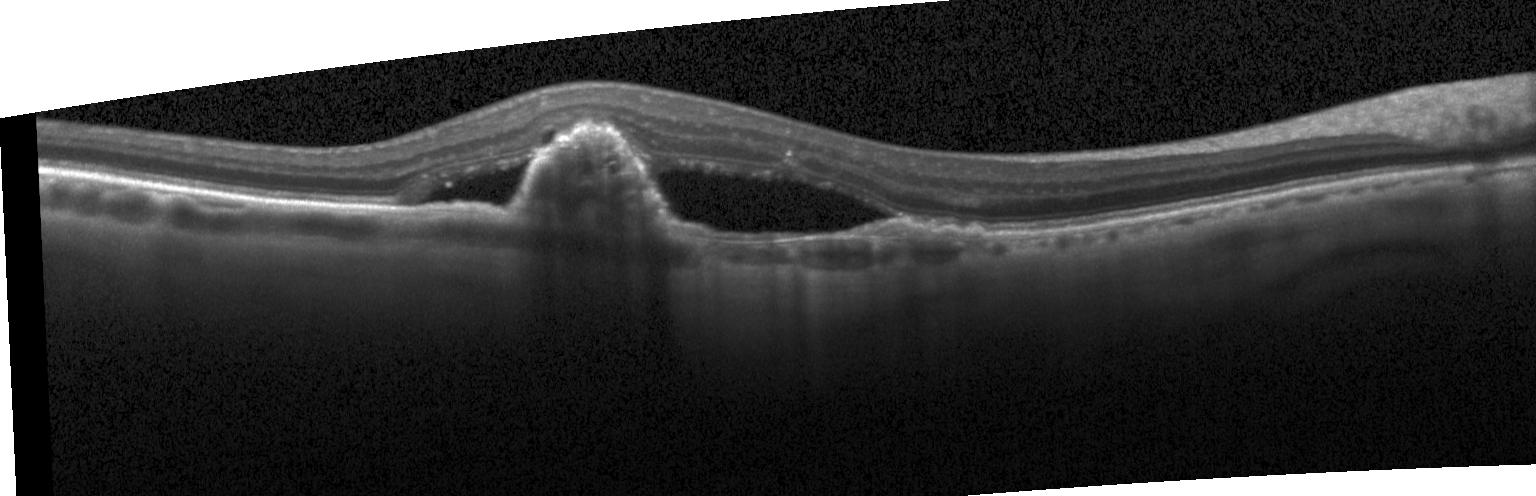
Impression: a choroidal neovascular membrane.